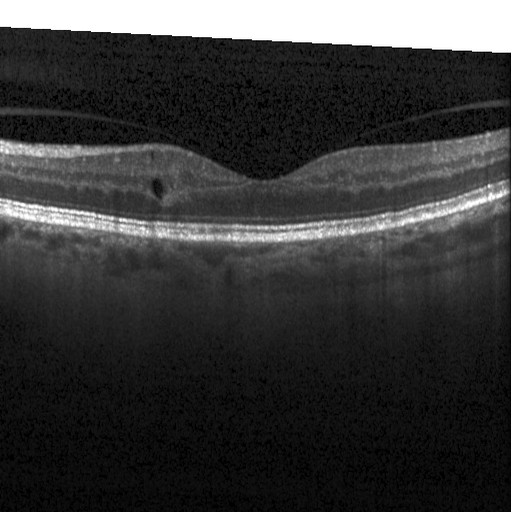 Fovea-centered, retinal OCT cross-section
OCT finding: DME.